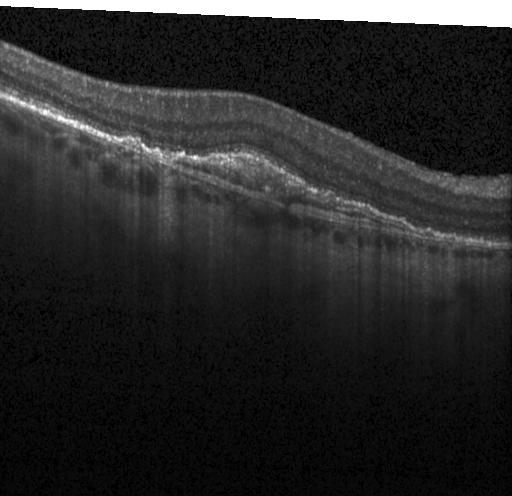 Spectral-domain OCT B-scan: a choroidal neovascular membrane.